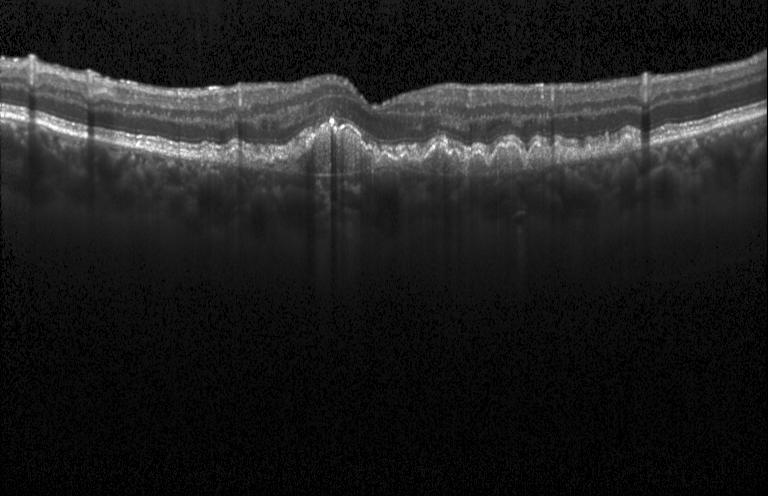
Retinal OCT cross-section · through the macula
Diagnosis: choroidal neovascularization.